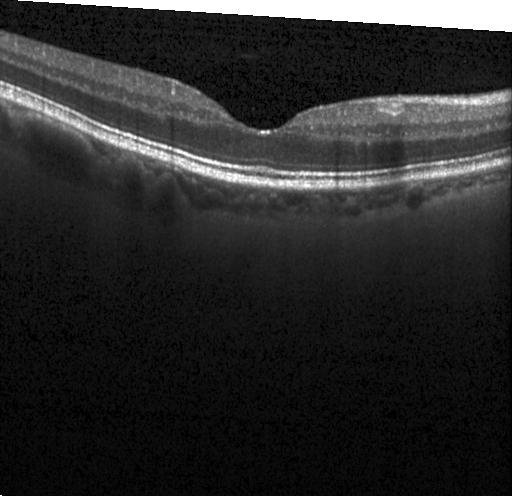

Heidelberg Spectralis, spectral-domain optical coherence tomography, OCT B-scan — The scan shows no CNV, no DME, and no drusen.